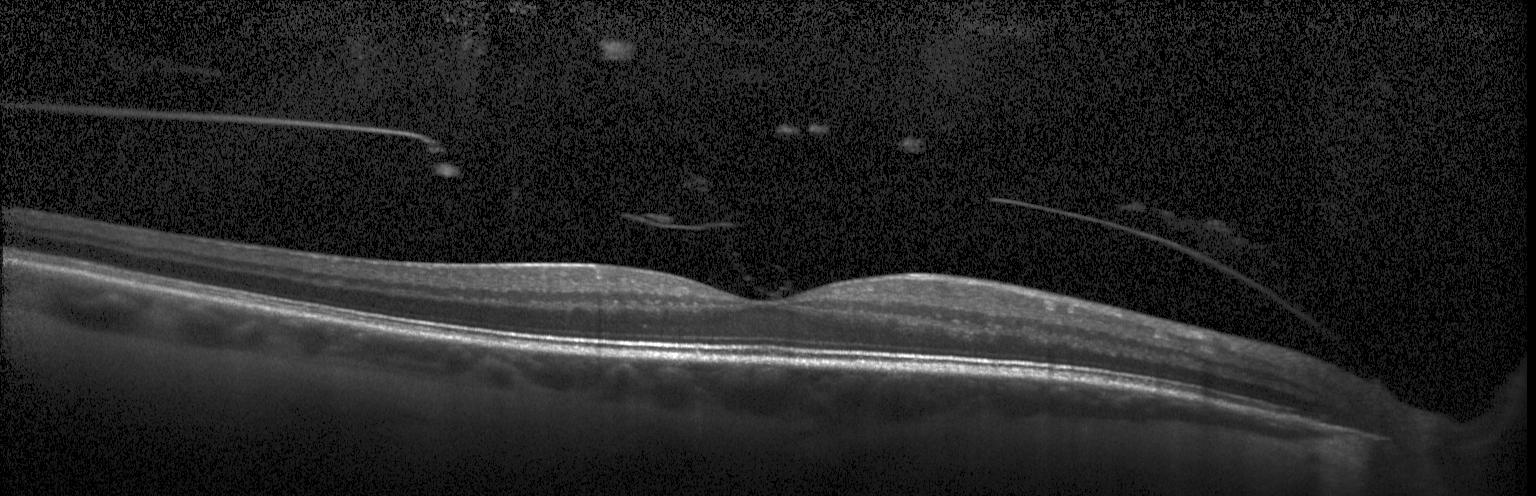 Assessment: neither choroidal neovascularization, diabetic macular edema, nor drusen.